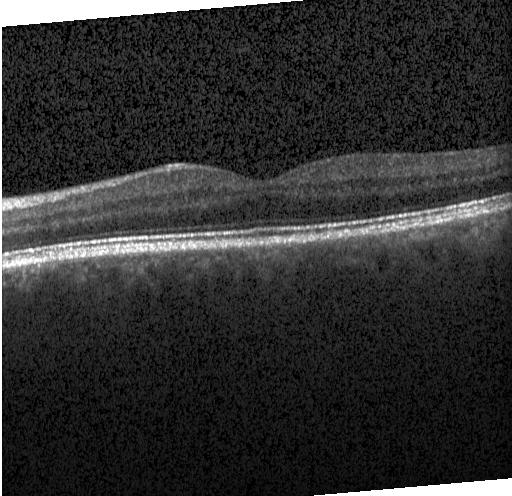

This B-scan demonstrates no evidence of CNV, DME, or drusen.